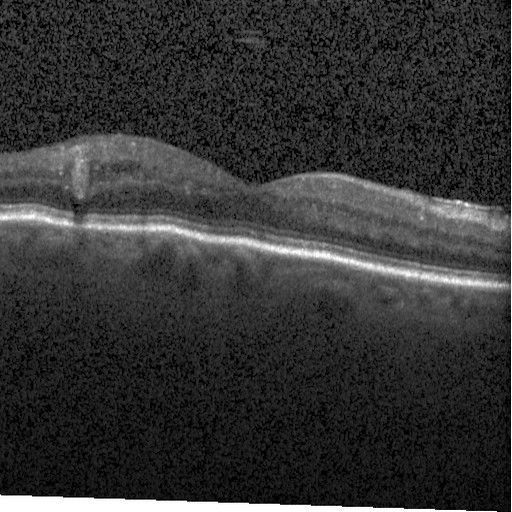
Heidelberg Spectralis · SD-OCT · retinal OCT cross-section — Assessment: DME.